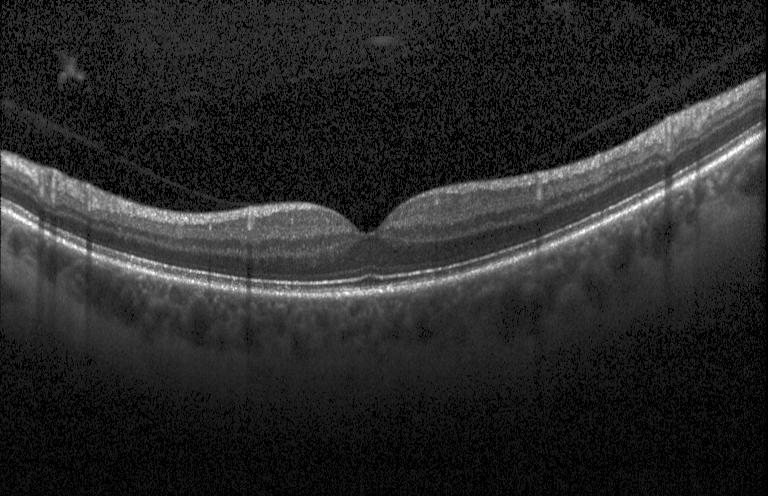 Spectral-domain optical coherence tomography, optical coherence tomography B-scan, acquired on a Heidelberg Spectralis, horizontal scan through the fovea.
Diagnosis: no CNV, no DME, and no drusen.